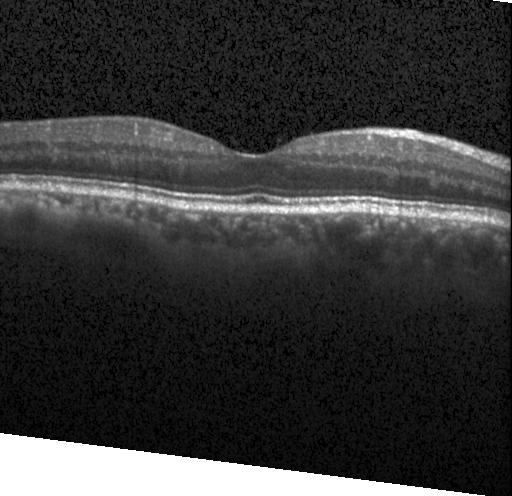 OCT line scan · through the macula.
Finding: no choroidal neovascularization, no diabetic macular edema, and no drusen.